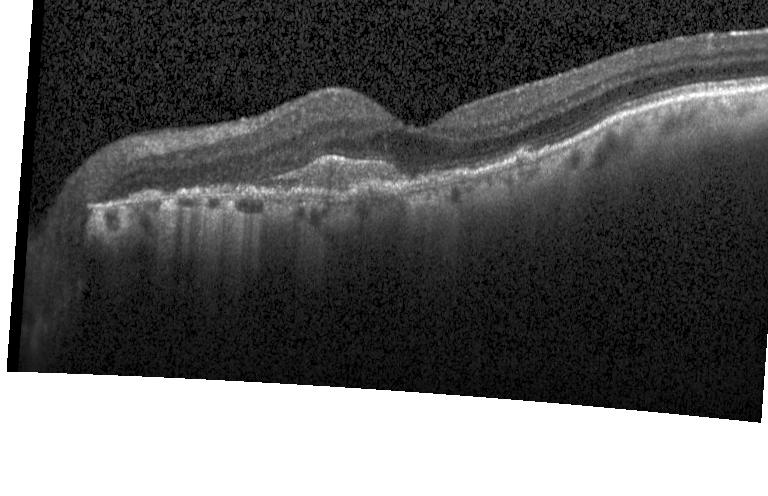

Horizontal scan through the fovea · retinal OCT cross-section · instrument: Heidelberg Spectralis
Diagnosis: a choroidal neovascular membrane.